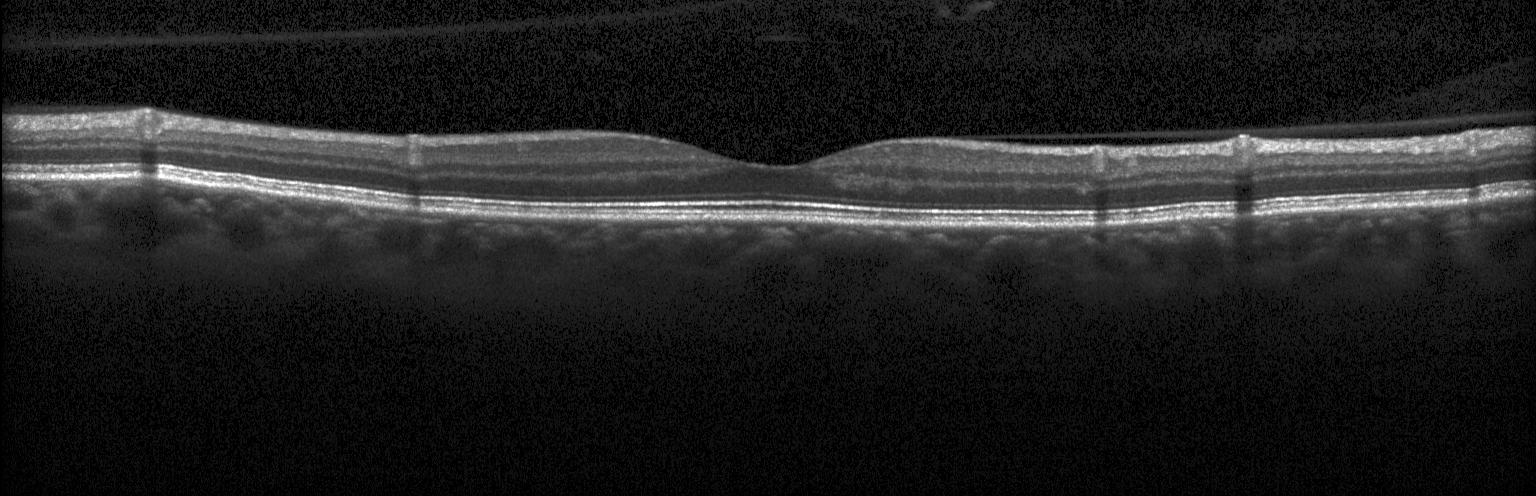

Heidelberg Spectralis. Optical coherence tomography scan. This B-scan demonstrates no evidence of choroidal neovascularization, diabetic macular edema, or drusen.